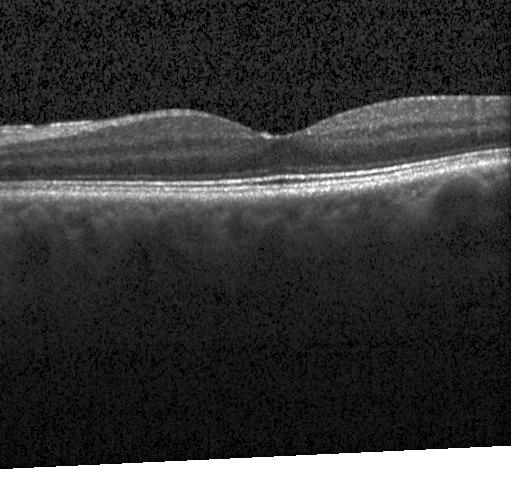 Horizontal scan through the fovea. OCT B-scan. SD-OCT. Assessment: neither choroidal neovascularization, diabetic macular edema, nor drusen.